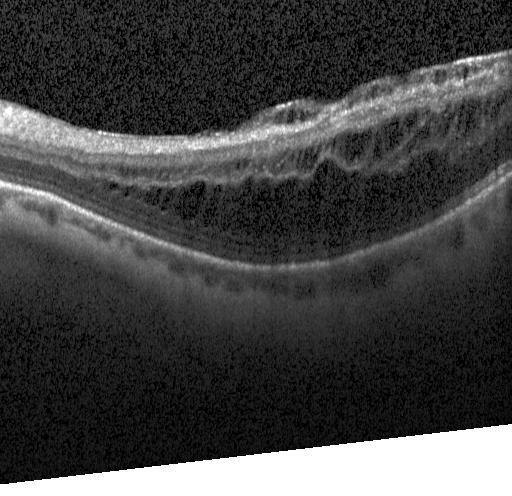
Optical coherence tomography B-scan; centered on the fovea; Heidelberg Spectralis OCT system. Dx: diabetic macular edema.